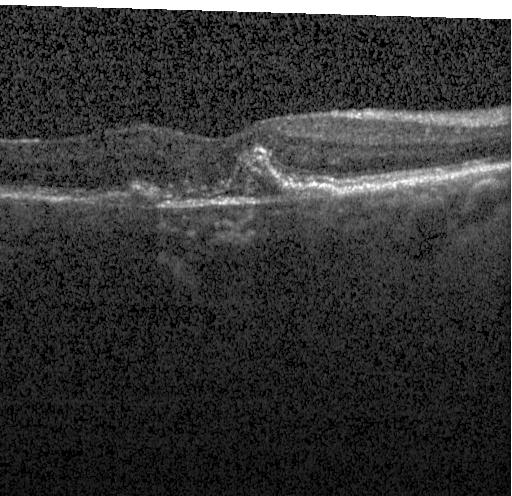

The scan shows CNV.